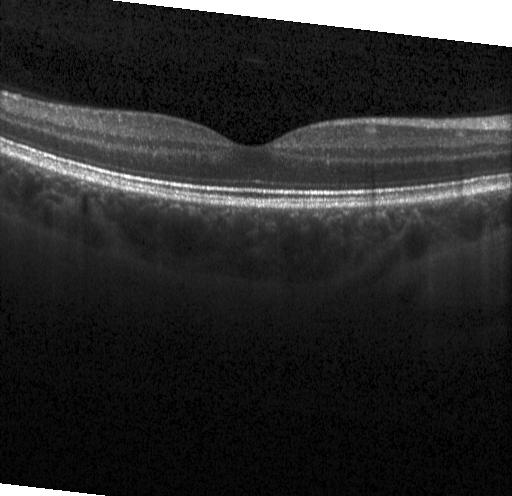
Finding: no choroidal neovascularization, diabetic macular edema, or drusen.